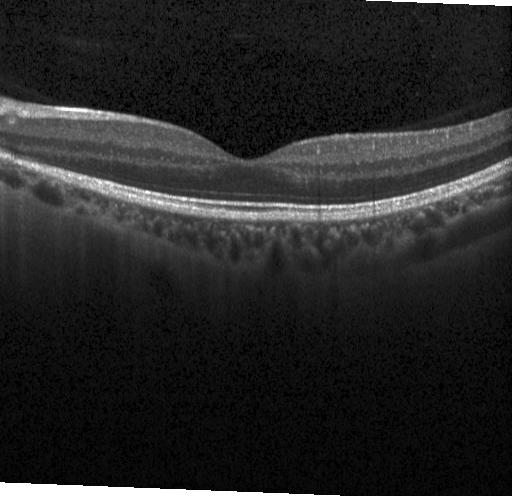

Spectral-domain optical coherence tomography; OCT line scan — Finding: neither choroidal neovascularization, diabetic macular edema, nor drusen.